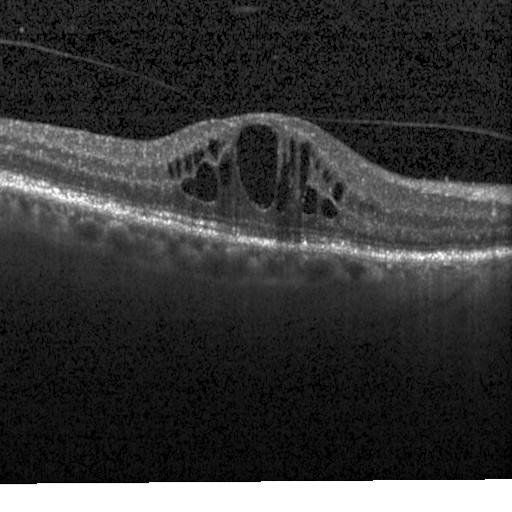

Optical coherence tomography scan
Assessment: diabetic macular edema.